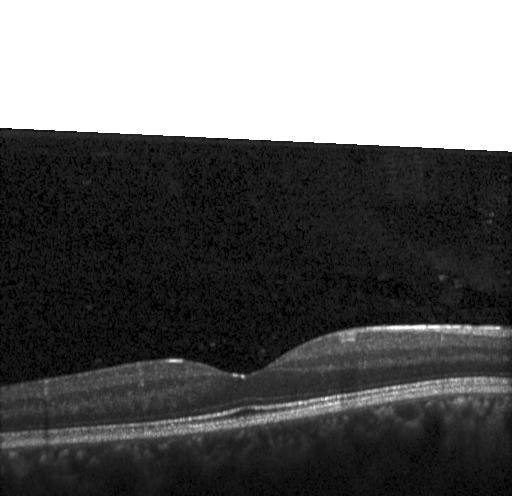

Impression: no choroidal neovascularization, no diabetic macular edema, and no drusen.